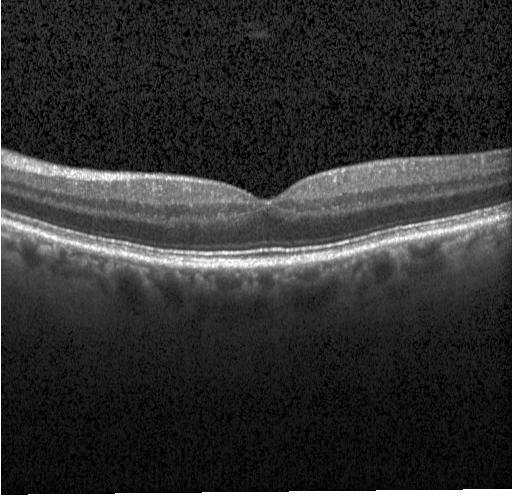

Retinal OCT cross-section — Impression: no choroidal neovascularization, no diabetic macular edema, and no drusen.